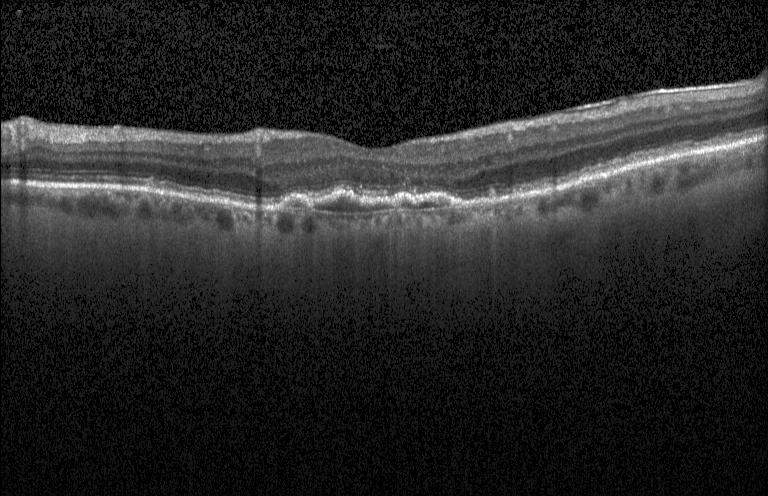
Impression: a choroidal neovascular membrane.